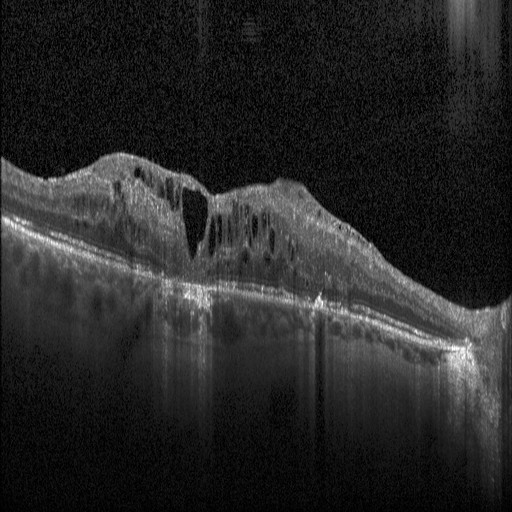

Optical coherence tomography scan.
Finding: diabetic macular edema.